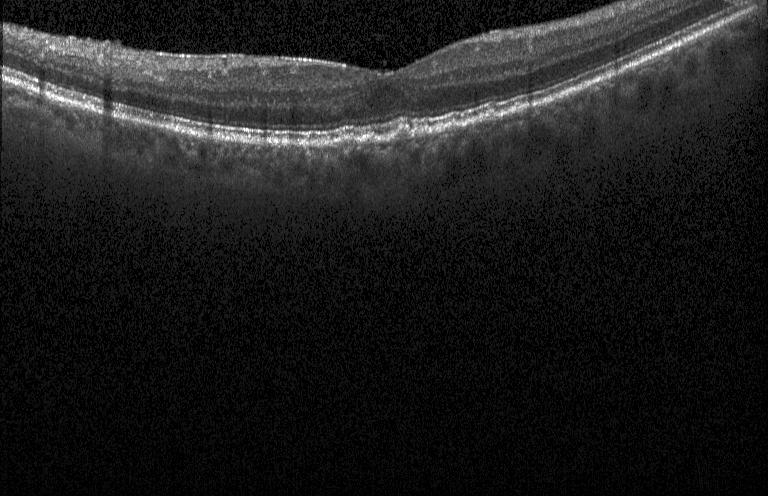 Optical coherence tomography scan, spectral-domain OCT
Impression: drusen.